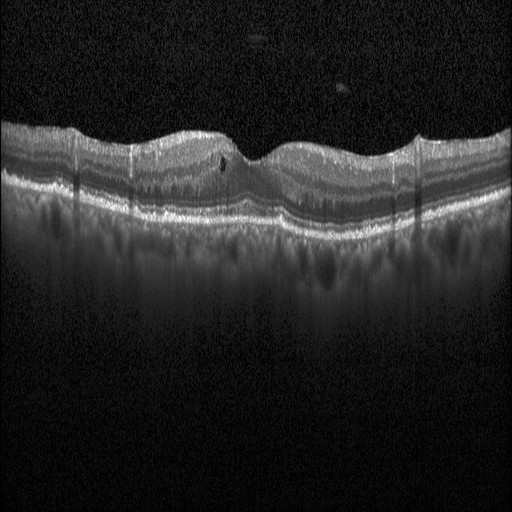
Spectral-domain OCT · macular scan · Heidelberg Spectralis · OCT line scan
Diagnosis: diabetic macular edema.